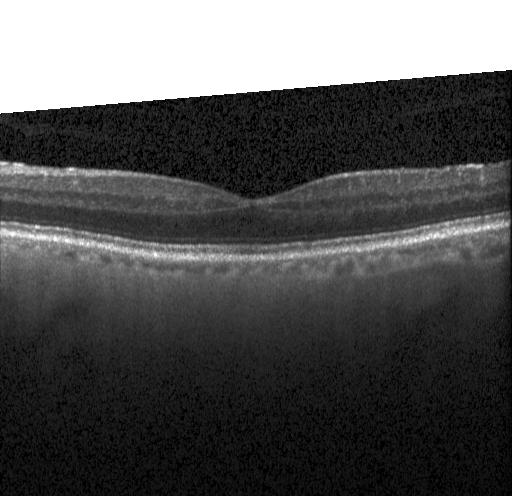
Macular OCT: no evidence of choroidal neovascularization, diabetic macular edema, or drusen.